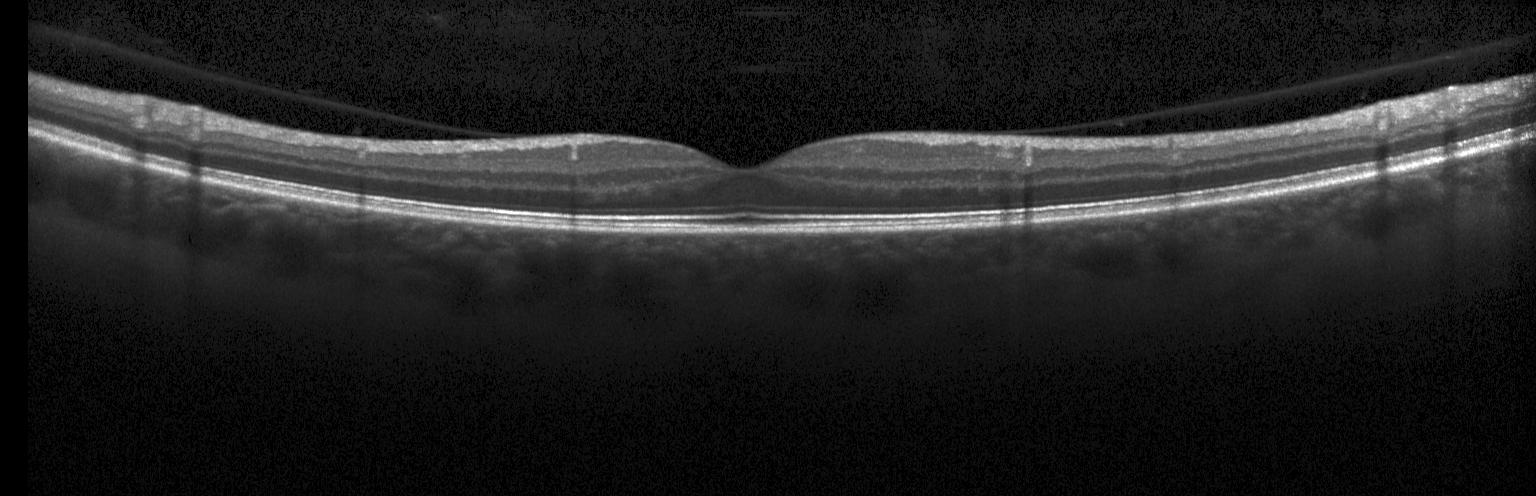

Heidelberg Spectralis, retinal OCT B-scan
Assessment: no CNV, no DME, and no drusen.